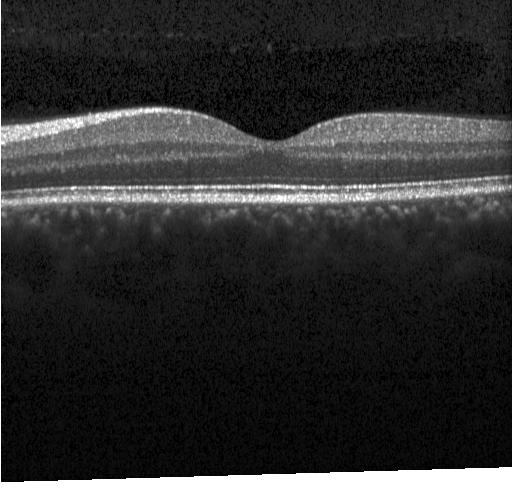 Instrument: Heidelberg Spectralis; OCT line scan; horizontal scan through the fovea
The scan shows no choroidal neovascularization, diabetic macular edema, or drusen.